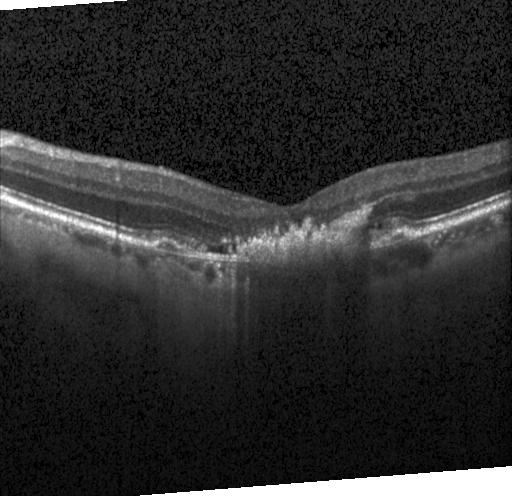
Impression: a choroidal neovascular membrane.